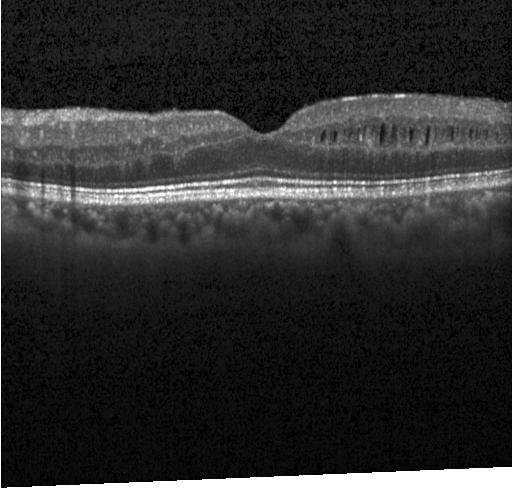
Macular OCT demonstrating diabetic macular edema (DME).